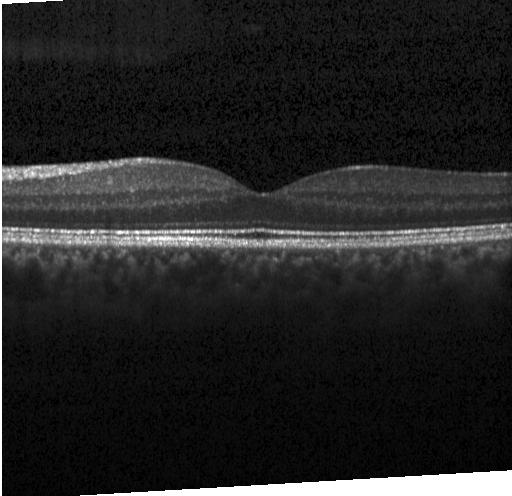 Impression: neither choroidal neovascularization, diabetic macular edema, nor drusen.